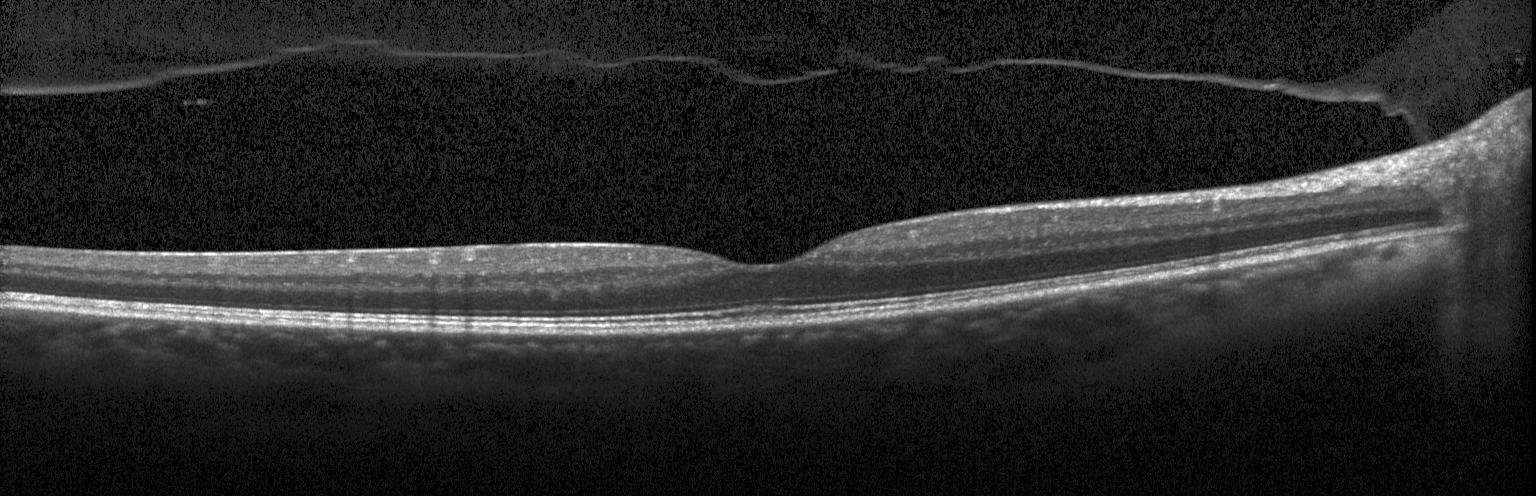
Assessment: no choroidal neovascularization, no diabetic macular edema, and no drusen.